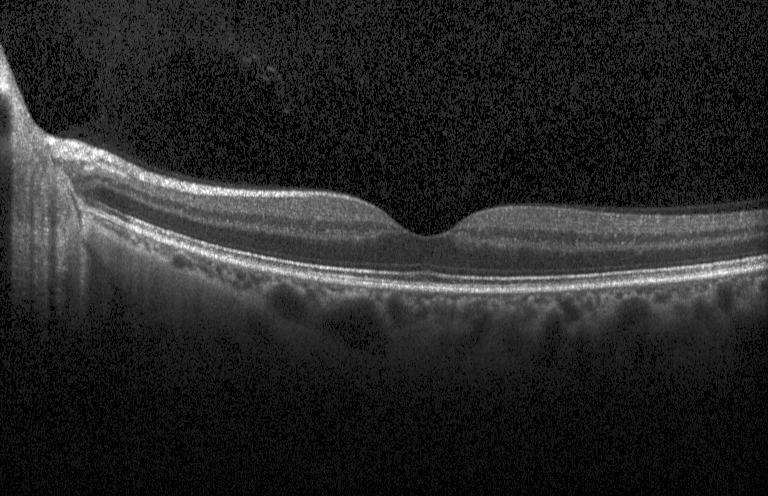
OCT finding: no evidence of choroidal neovascularization, diabetic macular edema, or drusen.